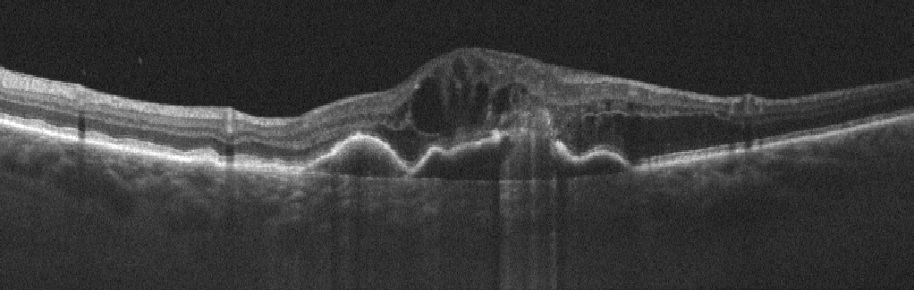
OCT scan showing age-related macular degeneration (AMD).